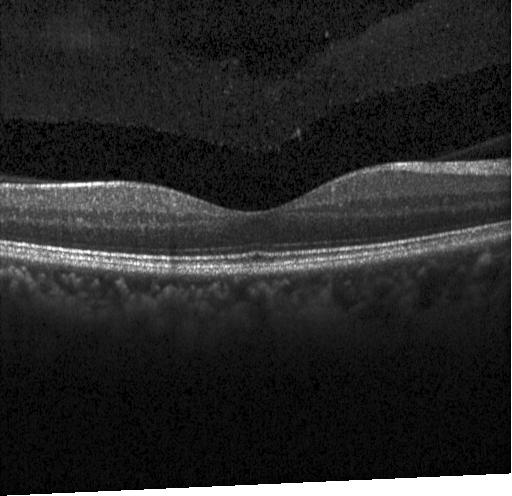
Optical coherence tomography B-scan, Heidelberg Spectralis OCT system, macular scan.
Assessment: neither CNV, DME, nor drusen.